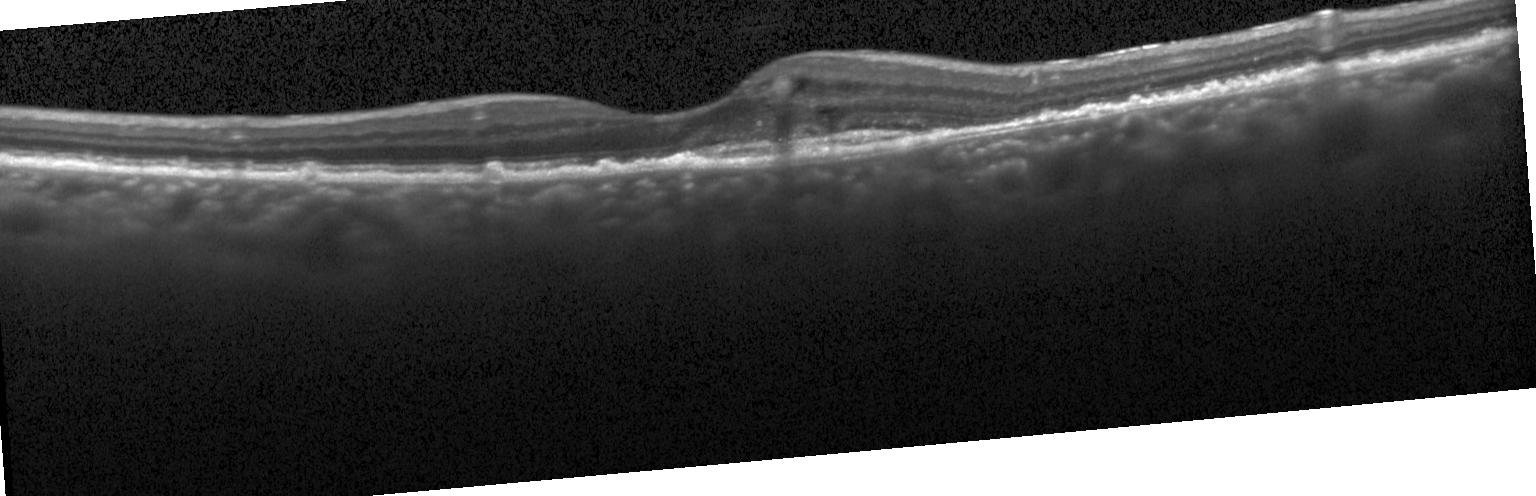
Retinal OCT B-scan
A choroidal neovascular membrane.